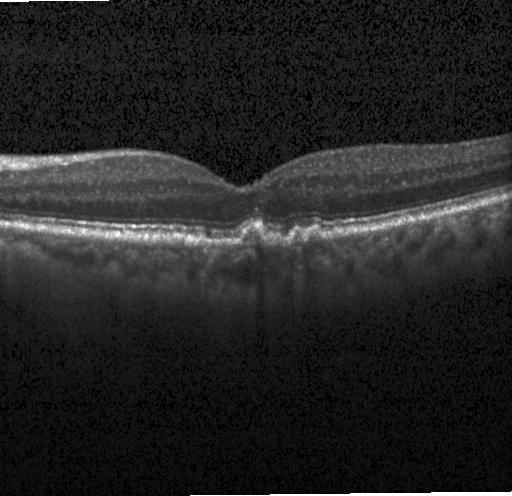 Spectral-domain OCT; acquired on a Heidelberg Spectralis; retinal OCT cross-section; horizontal scan through the fovea. OCT finding: drusen.